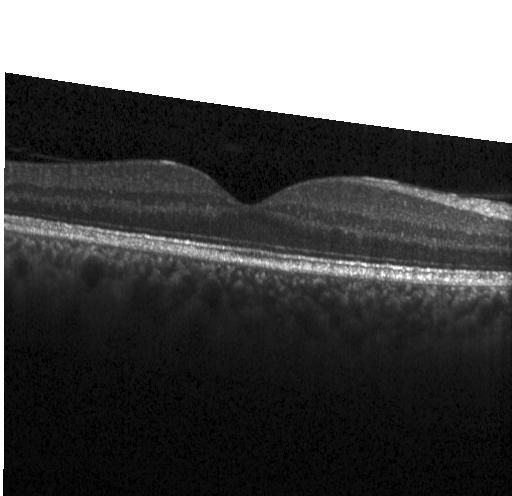 Diagnosis: no choroidal neovascularization, diabetic macular edema, or drusen.